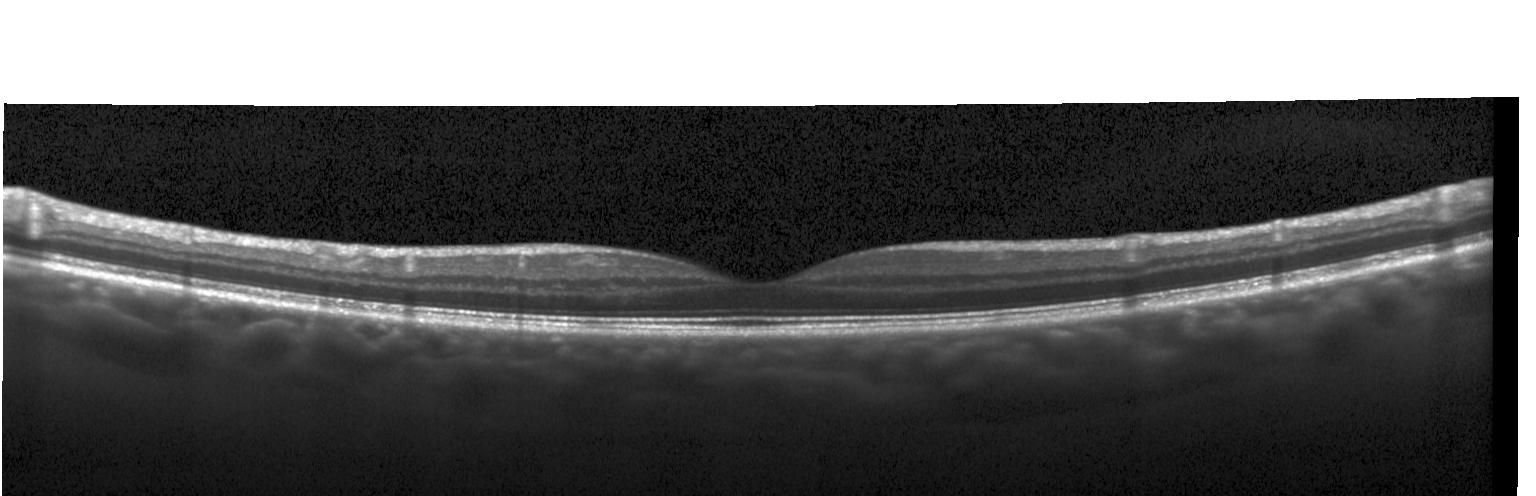 Spectral-domain optical coherence tomography · optical coherence tomography scan · through the macula · Heidelberg Spectralis — No evidence of choroidal neovascularization, diabetic macular edema, or drusen.